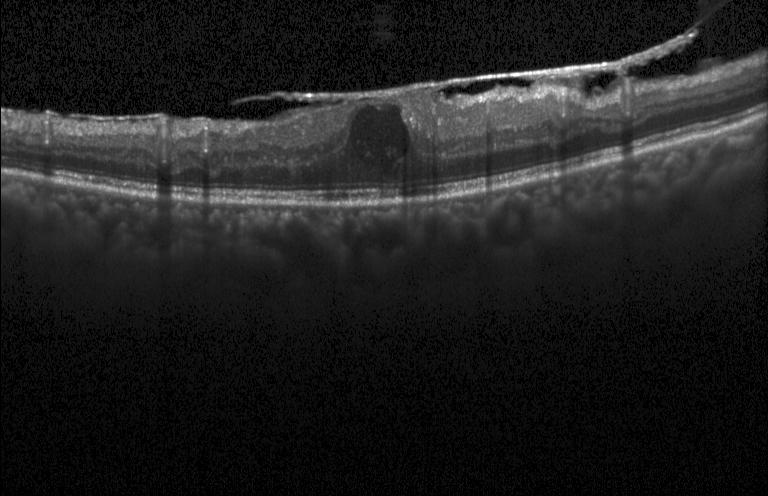

Macular OCT demonstrating diabetic macular edema (DME).